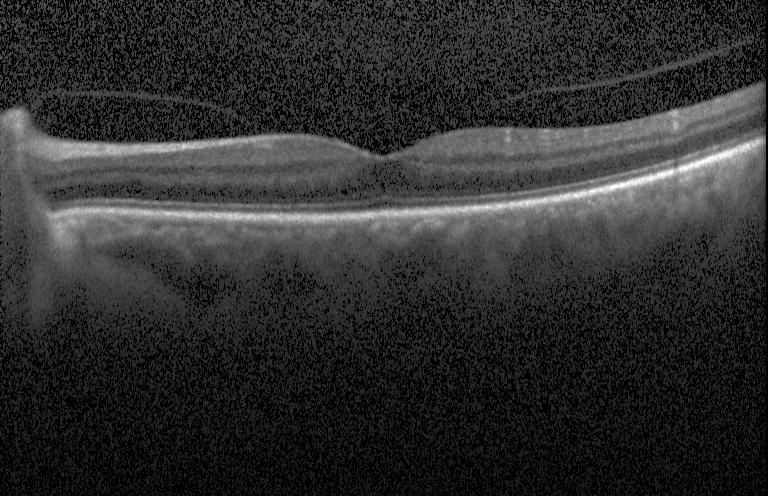 Retinal OCT cross-section showing no choroidal neovascularization, diabetic macular edema, or drusen.